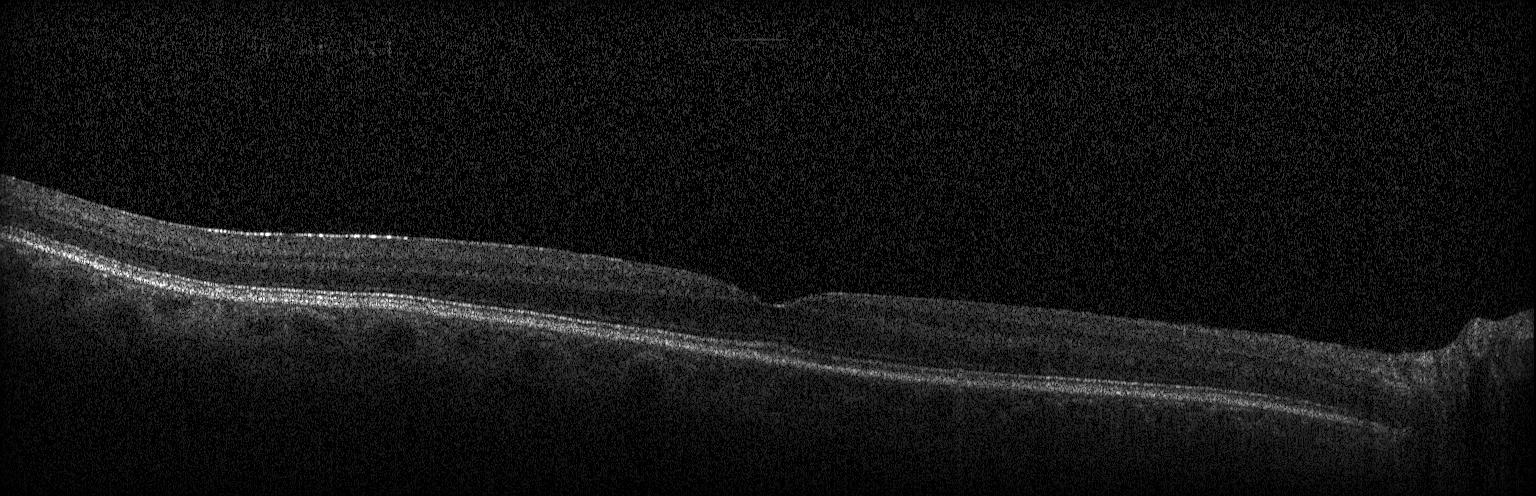
OCT B-scan
Impression: no choroidal neovascularization, diabetic macular edema, or drusen.